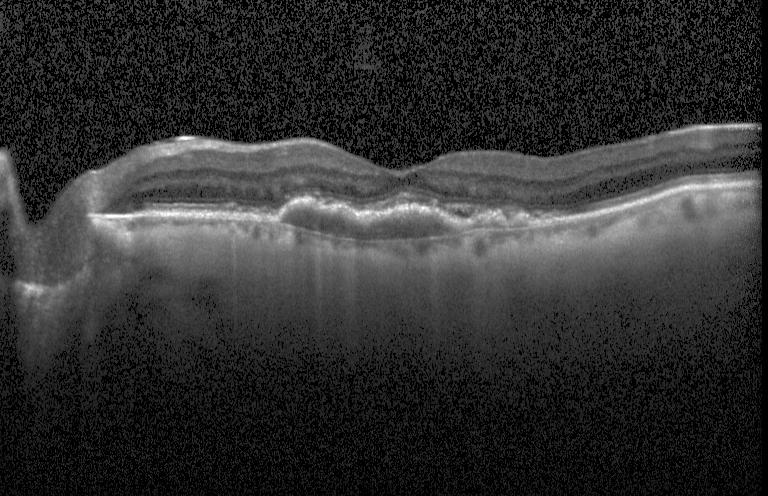 Spectral-domain optical coherence tomography. Centered on the fovea. Heidelberg Spectralis. OCT line scan — This B-scan demonstrates a choroidal neovascular membrane.